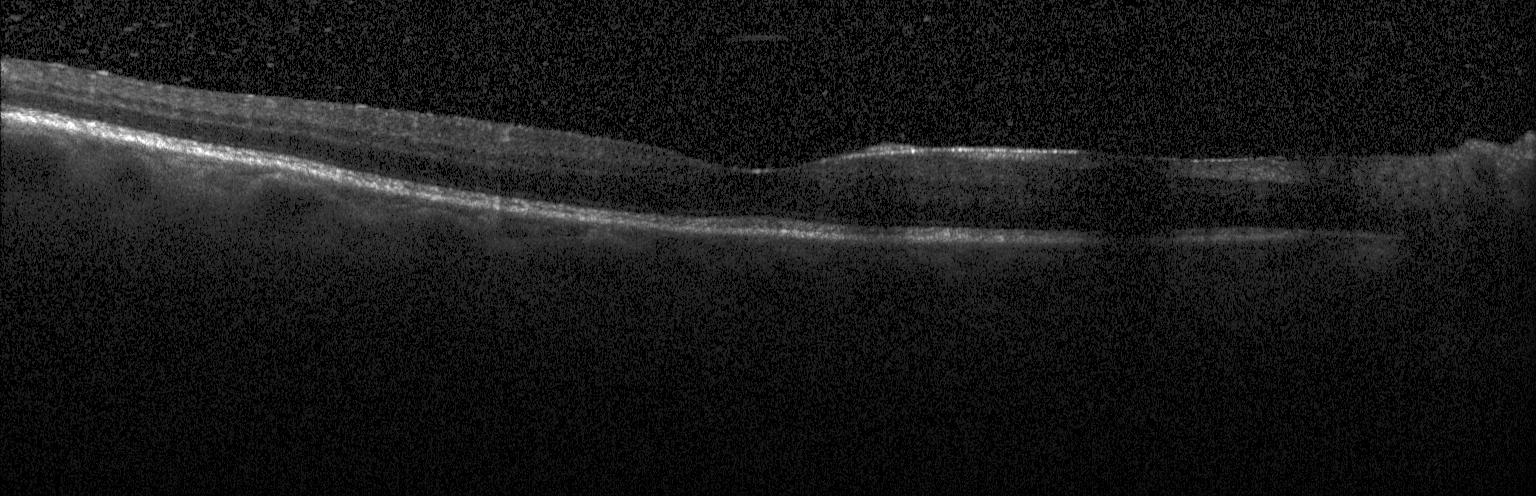
Impression: no evidence of CNV, DME, or drusen.